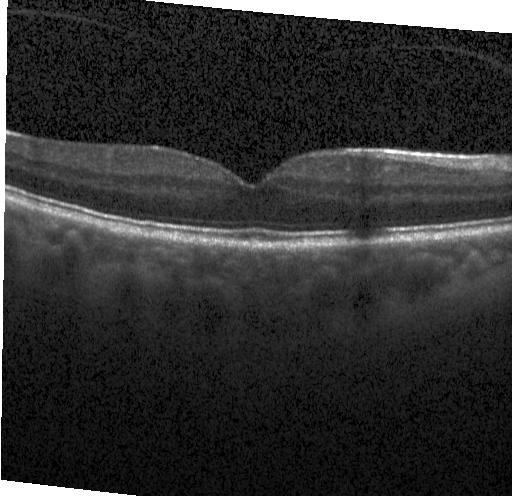 SD-OCT. Instrument: Heidelberg Spectralis. Retinal OCT cross-section — Diagnosis: neither CNV, DME, nor drusen.